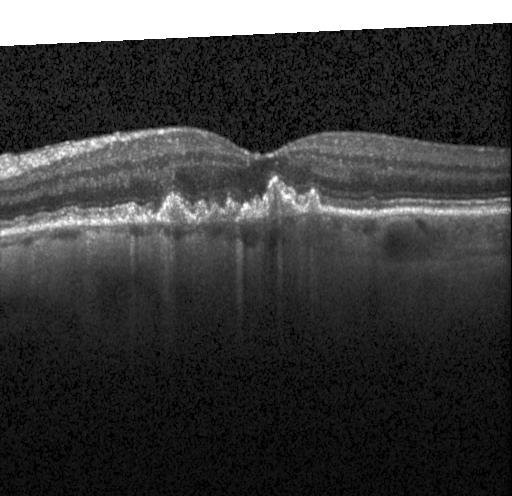
This B-scan demonstrates drusen.